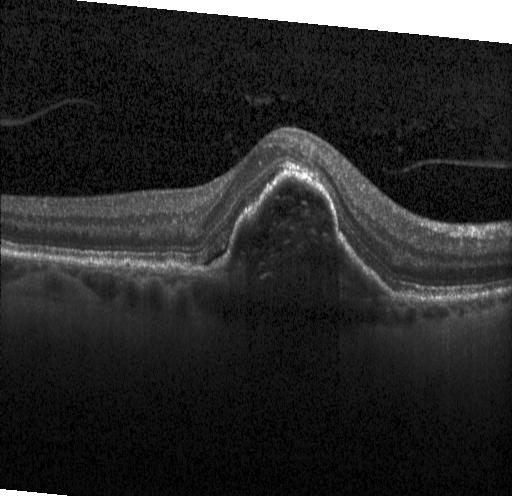

Retinal OCT cross-section, SD-OCT, through the macula
Choroidal neovascularization.